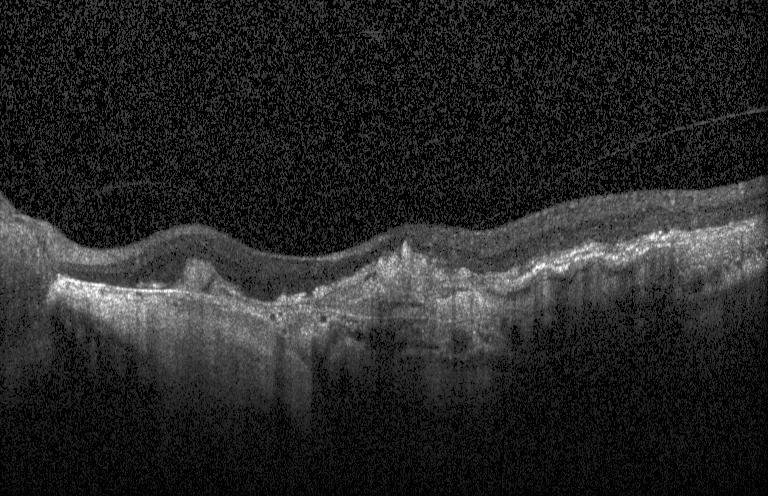
OCT B-scan showing choroidal neovascularization.